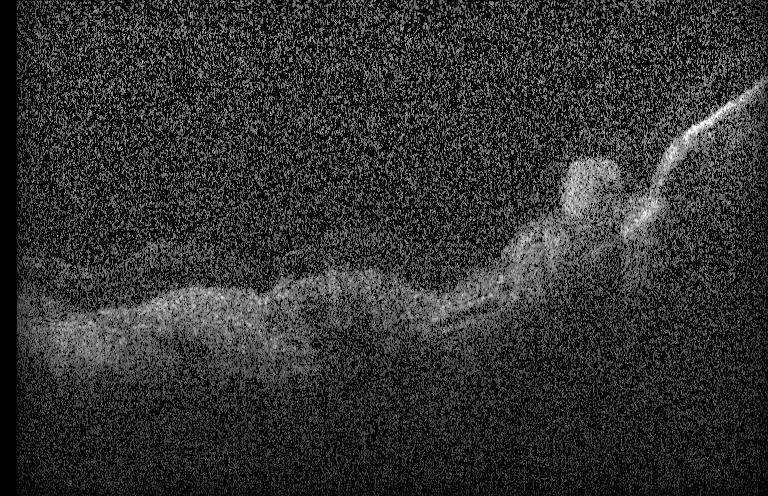

Retinal OCT cross-section showing CNV.